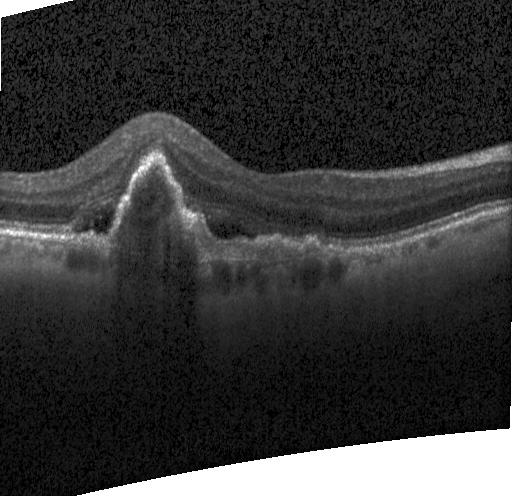
SD-OCT, OCT line scan — The scan shows a choroidal neovascular membrane.